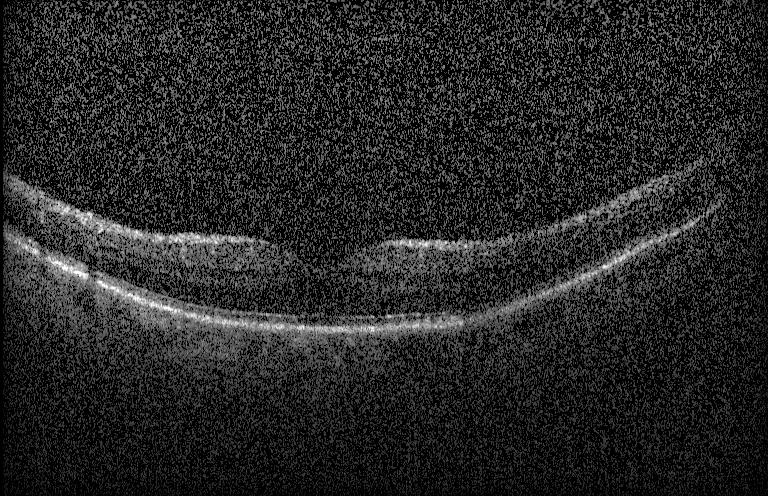
Heidelberg Spectralis OCT system · SD-OCT · OCT line scan · fovea-centered
Impression: neither choroidal neovascularization, diabetic macular edema, nor drusen.